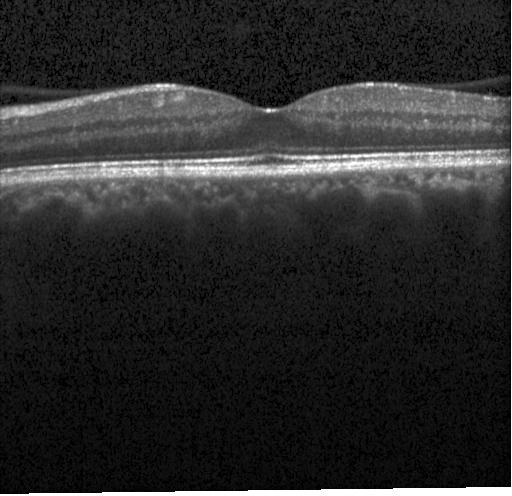 Macular OCT: no choroidal neovascularization, diabetic macular edema, or drusen.